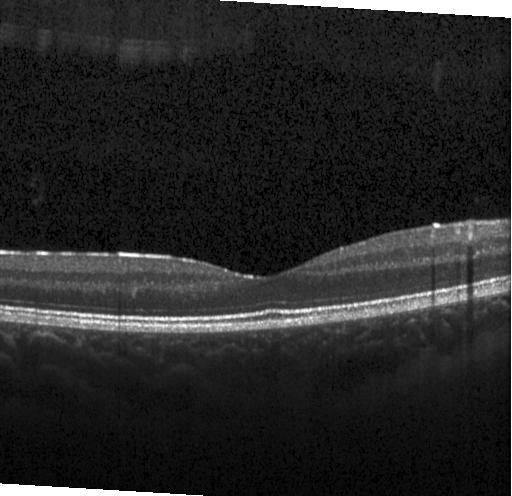
Fovea-centered. Instrument: Heidelberg Spectralis. Retinal OCT B-scan — Diagnosis: no evidence of choroidal neovascularization, diabetic macular edema, or drusen.